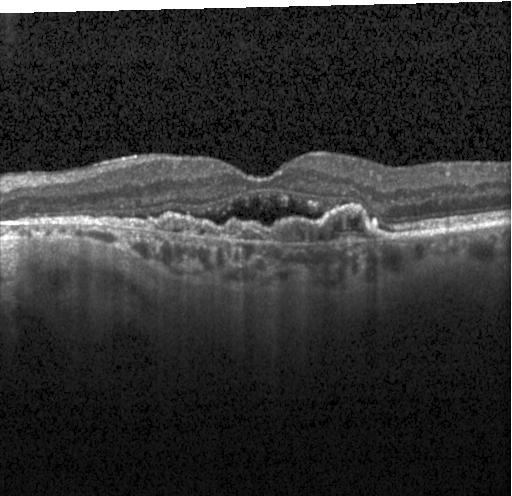
Optical coherence tomography B-scan; Heidelberg Spectralis OCT system
This B-scan demonstrates CNV.